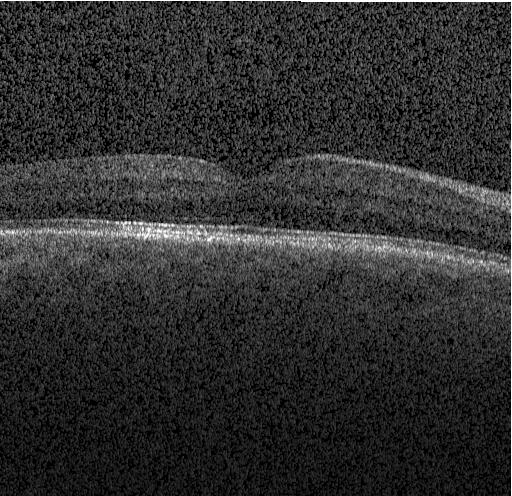 Acquired on a Heidelberg Spectralis · SD-OCT · retinal OCT B-scan
The scan shows no choroidal neovascularization, diabetic macular edema, or drusen.